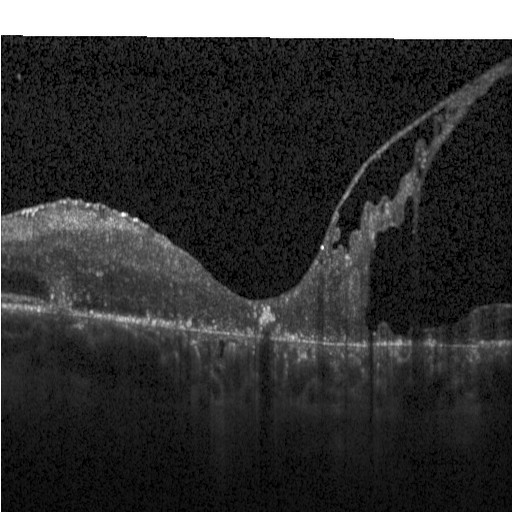 Instrument: Heidelberg Spectralis, optical coherence tomography scan — Finding: DME.